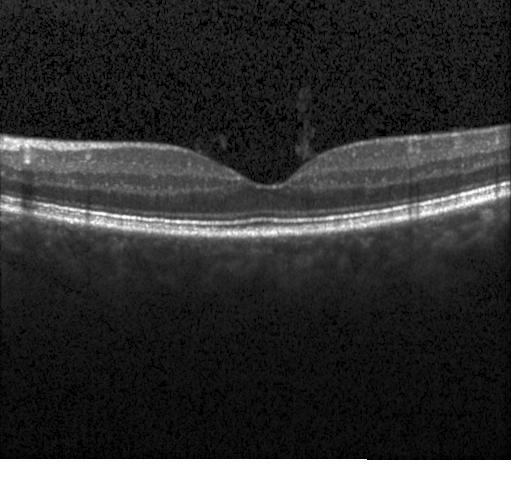 Optical coherence tomography B-scan · through the macula · spectral-domain optical coherence tomography · acquired on a Heidelberg Spectralis
This B-scan demonstrates no choroidal neovascularization, diabetic macular edema, or drusen.